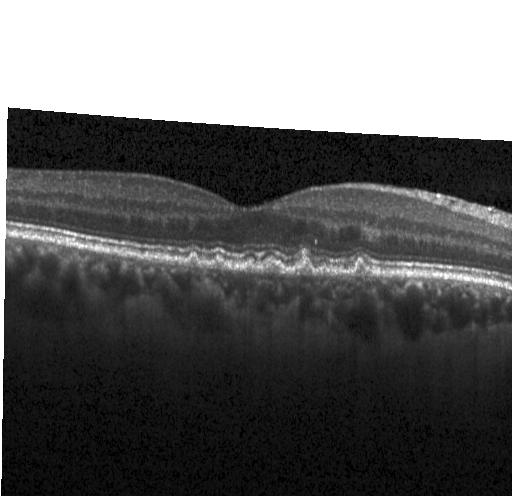

Centered on the fovea. Retinal OCT cross-section. Spectral-domain OCT. Heidelberg Spectralis. This B-scan demonstrates multiple drusen.